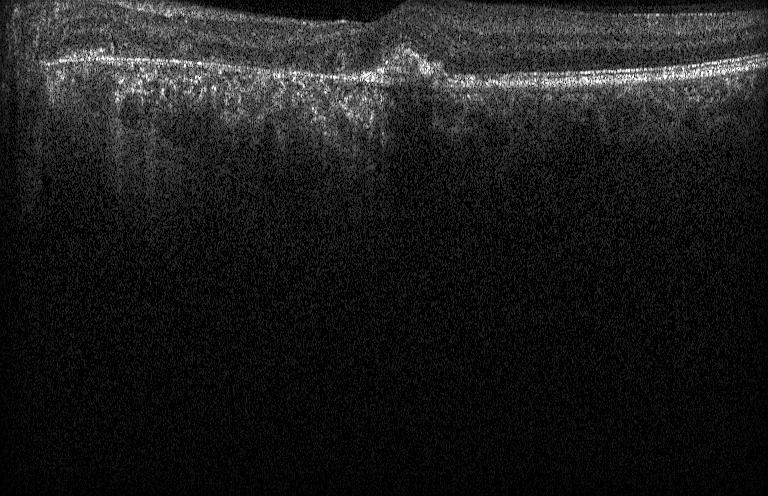
This B-scan demonstrates a choroidal neovascular membrane.